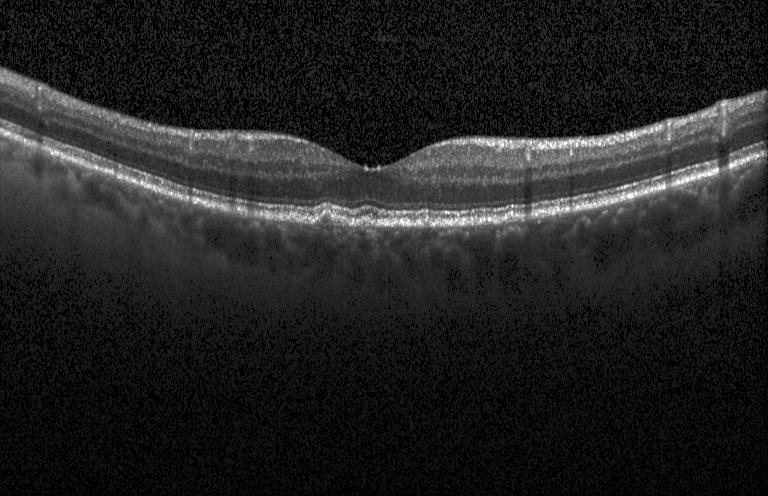
OCT finding: multiple drusen.